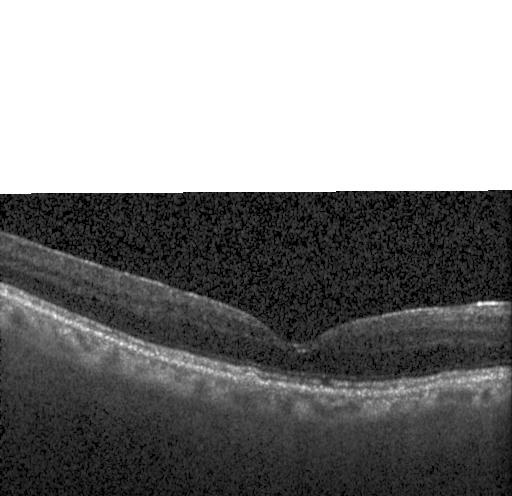

Horizontal scan through the fovea. Heidelberg Spectralis. Spectral-domain optical coherence tomography. Retinal OCT B-scan
No evidence of choroidal neovascularization, diabetic macular edema, or drusen.